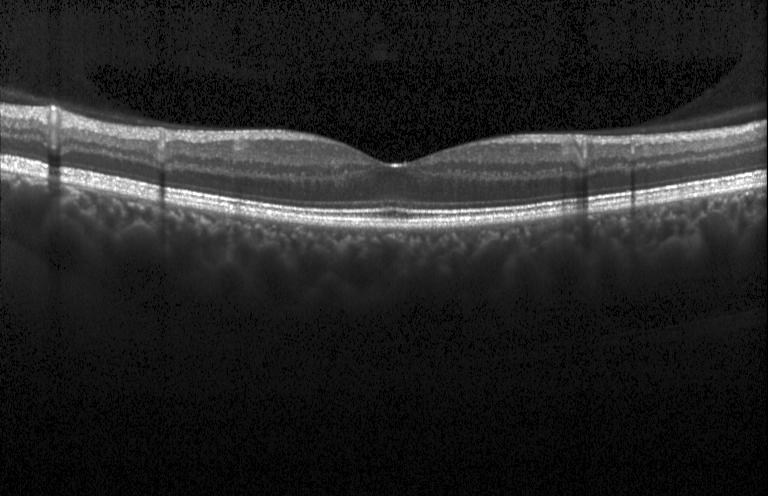 OCT B-scan showing no choroidal neovascularization, no diabetic macular edema, and no drusen.